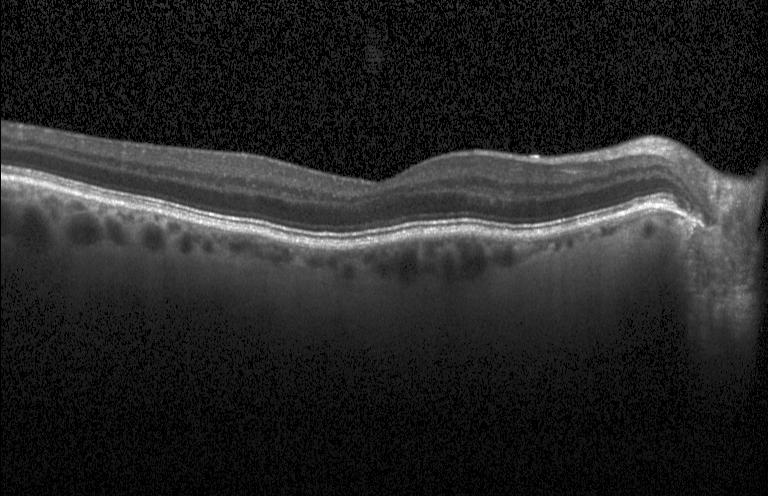 The scan shows neither CNV, DME, nor drusen.